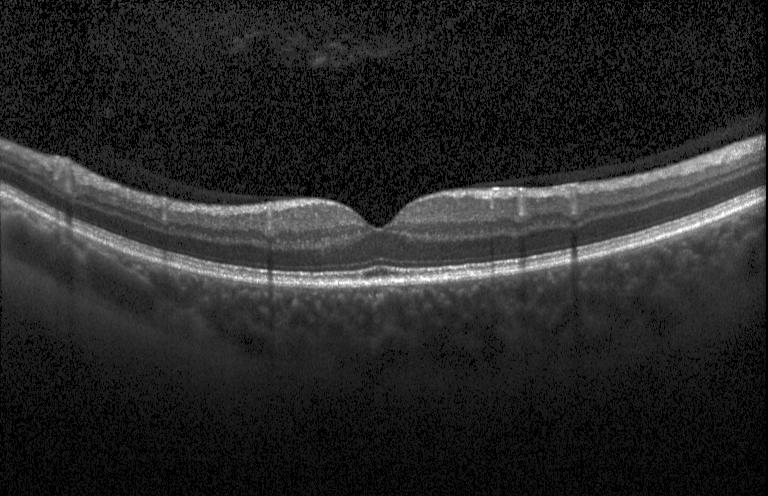 OCT scan showing no CNV, no DME, and no drusen.